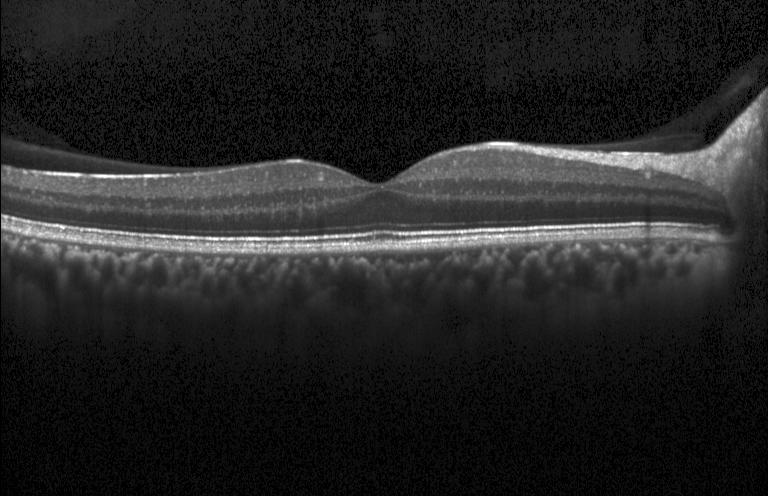 Finding: no choroidal neovascularization, diabetic macular edema, or drusen.